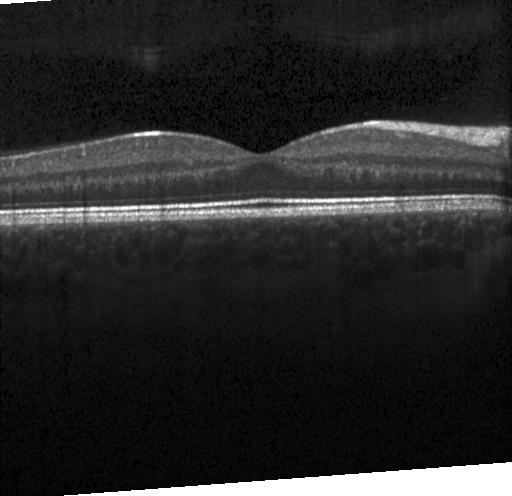 Spectral-domain OCT, OCT line scan
This B-scan demonstrates neither CNV, DME, nor drusen.